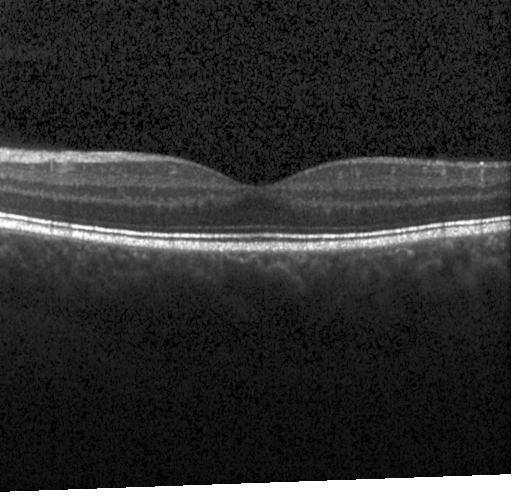

SD-OCT; horizontal scan through the fovea; retinal OCT cross-section; acquired on a Heidelberg Spectralis
Impression: no choroidal neovascularization, diabetic macular edema, or drusen.